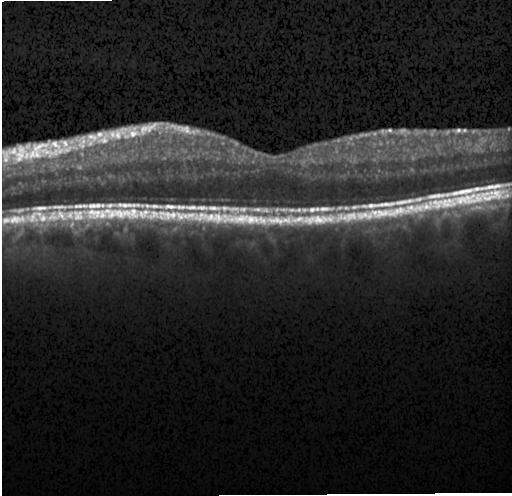 Retinal OCT B-scan. Spectral-domain optical coherence tomography — Diagnosis: neither choroidal neovascularization, diabetic macular edema, nor drusen.